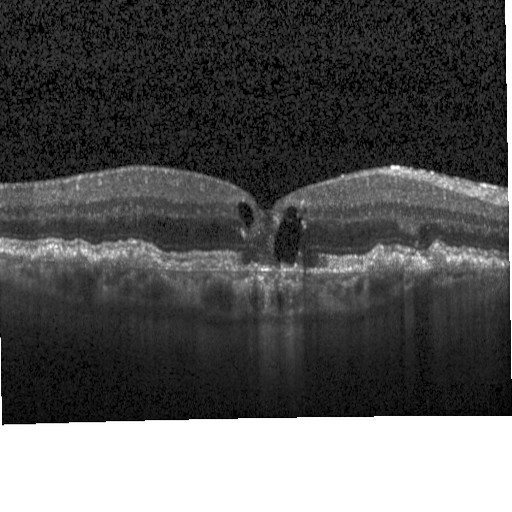
Acquired on a Heidelberg Spectralis · SD-OCT · OCT B-scan · centered on the fovea — Finding: DME.